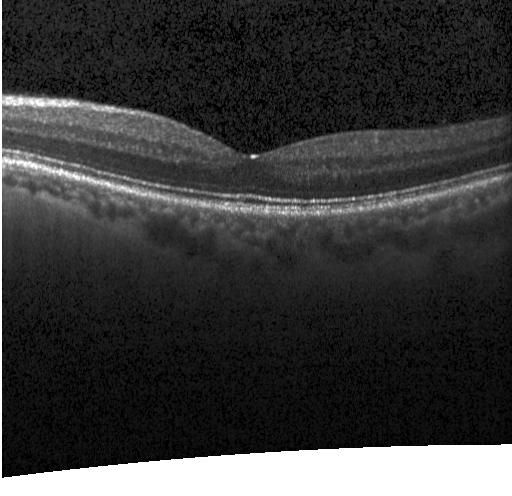

OCT B-scan.
Dx: no choroidal neovascularization, no diabetic macular edema, and no drusen.